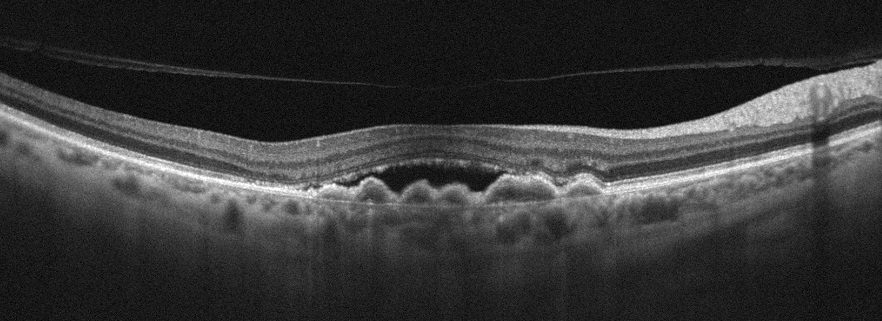 Optical coherence tomography B-scan.
OCT finding: age-related macular degeneration (AMD).